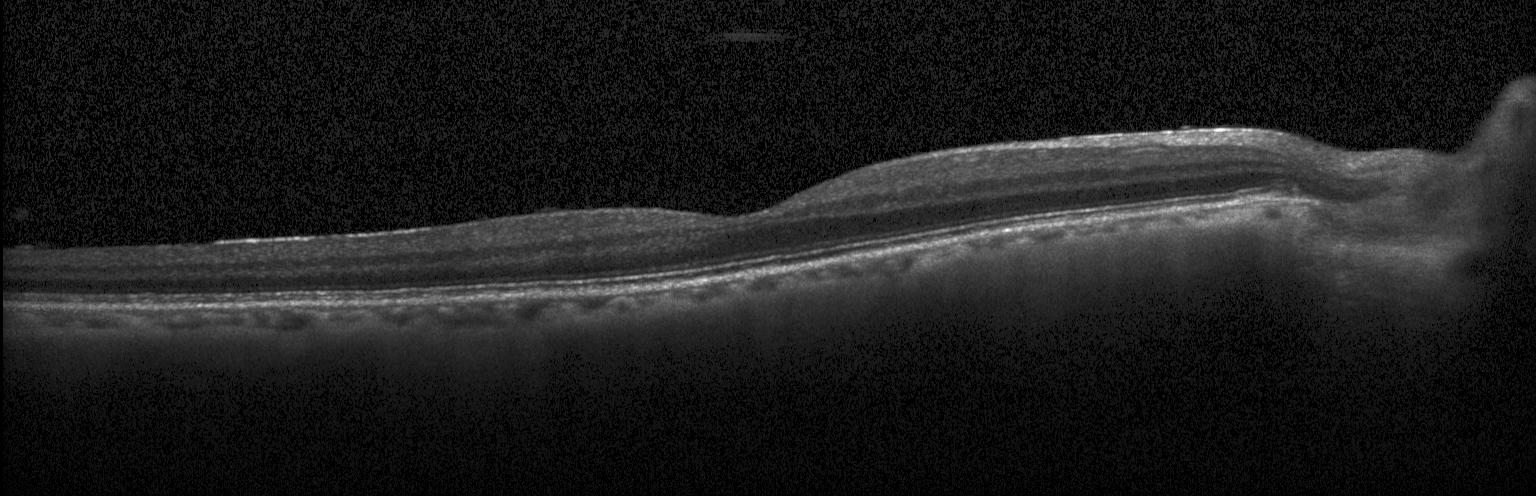
OCT B-scan; SD-OCT; instrument: Heidelberg Spectralis
Neither CNV, DME, nor drusen.